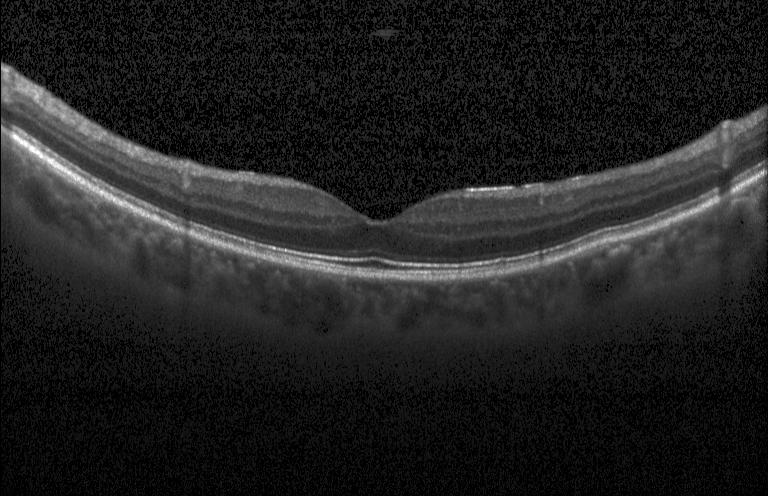 Spectral-domain OCT. Retinal OCT B-scan. Macular scan. Instrument: Heidelberg Spectralis.
This B-scan demonstrates no evidence of choroidal neovascularization, diabetic macular edema, or drusen.